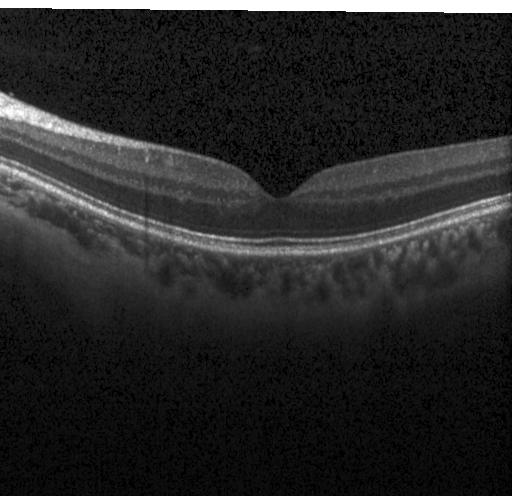 SD-OCT. Optical coherence tomography scan — Assessment: neither CNV, DME, nor drusen.